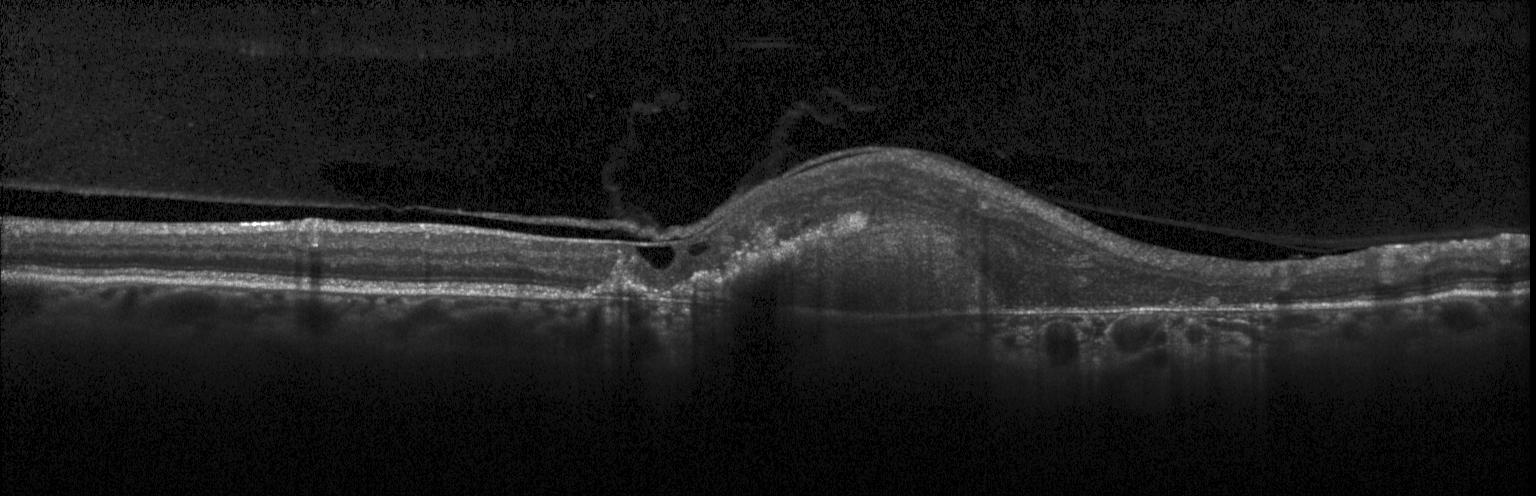

Dx: a choroidal neovascular membrane.